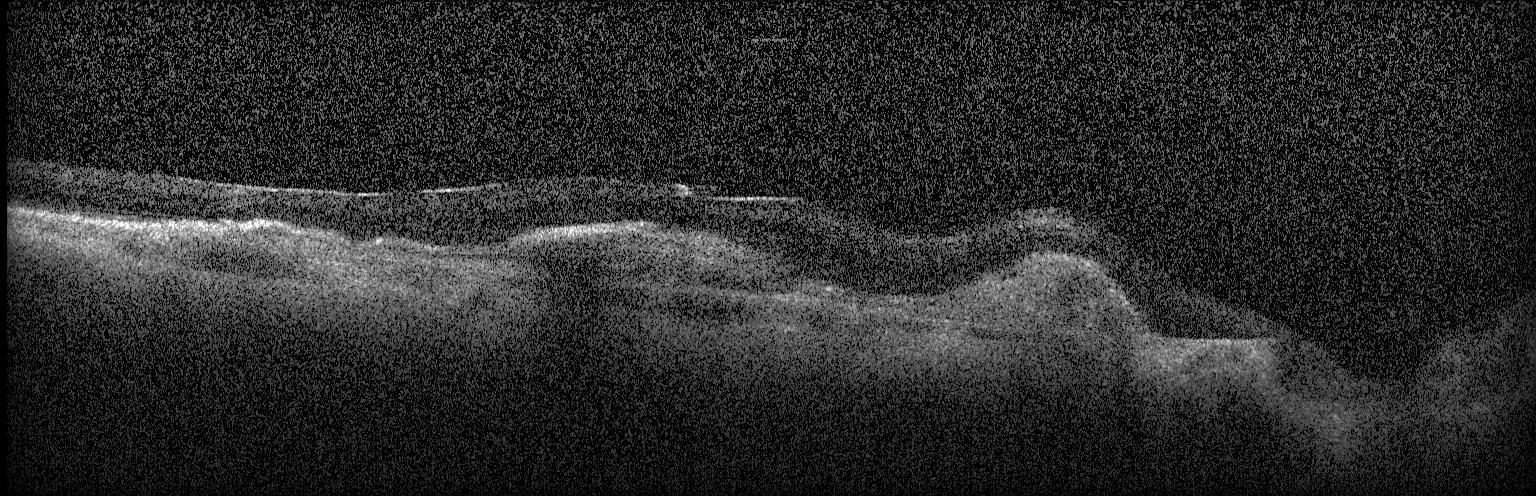 Diagnosis: a choroidal neovascular membrane.